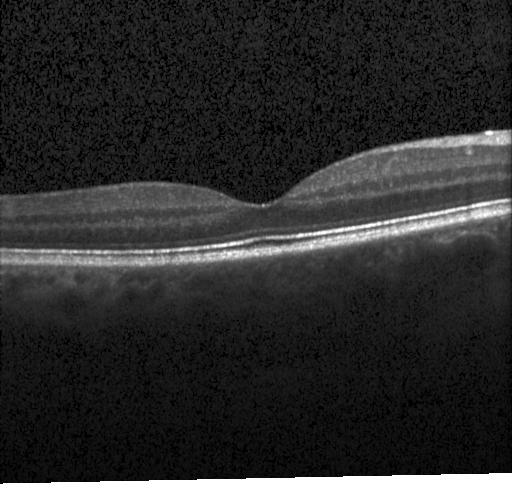
This B-scan demonstrates neither CNV, DME, nor drusen.